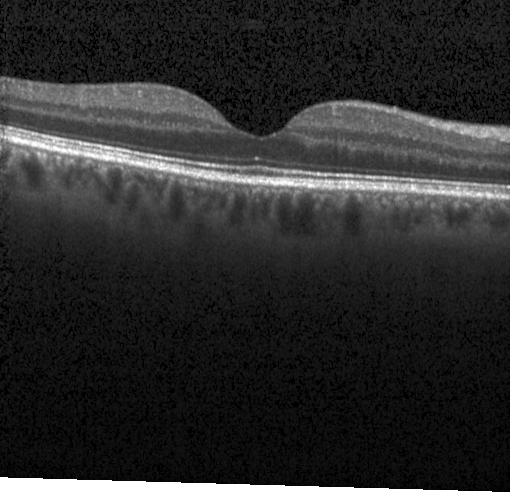

Finding: no choroidal neovascularization, diabetic macular edema, or drusen.